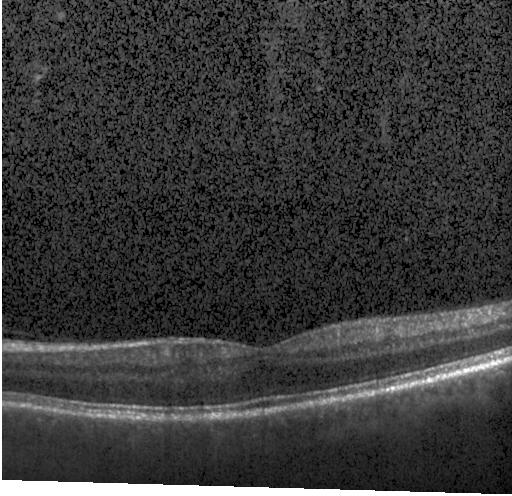
Macular OCT: no CNV, no DME, and no drusen.